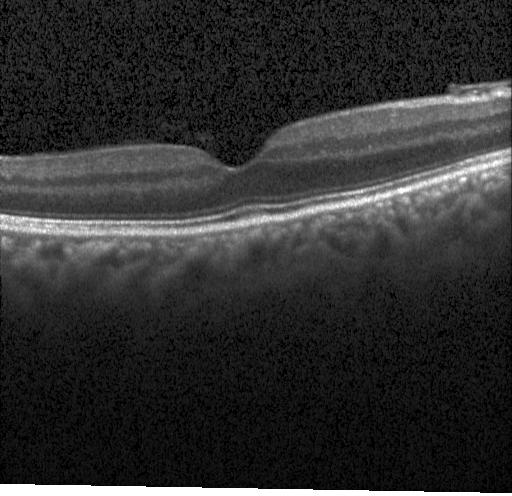

Fovea-centered · optical coherence tomography B-scan. Finding: no CNV, DME, or drusen.